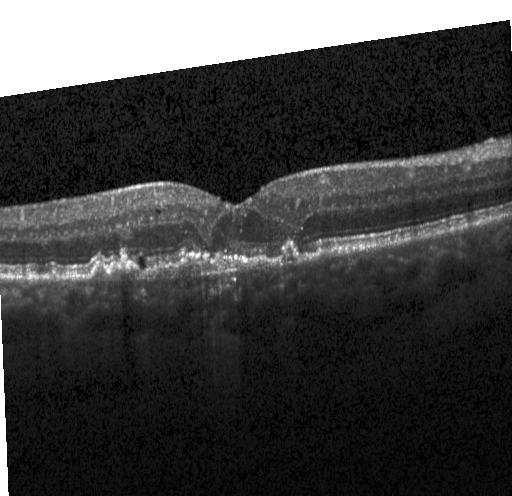
Spectral-domain OCT; OCT line scan. This B-scan demonstrates a choroidal neovascular membrane.